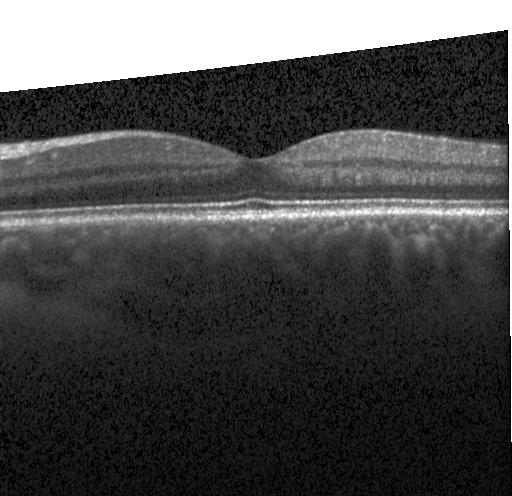 No choroidal neovascularization, diabetic macular edema, or drusen.